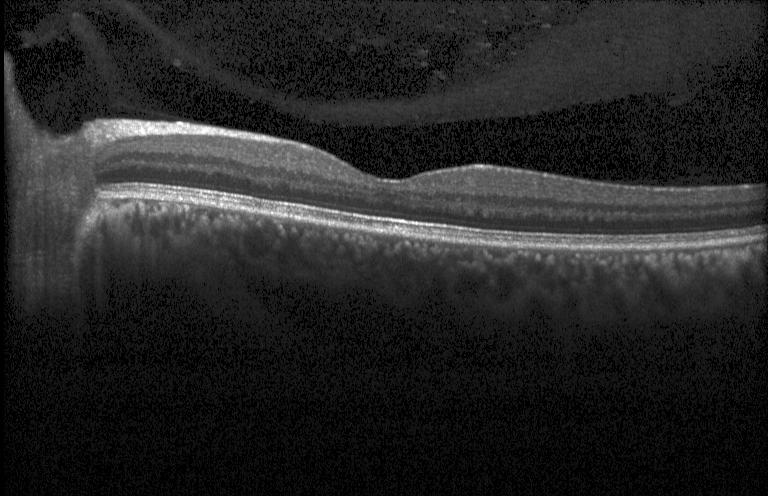 Fovea-centered · optical coherence tomography scan.
Macular OCT: no CNV, DME, or drusen.